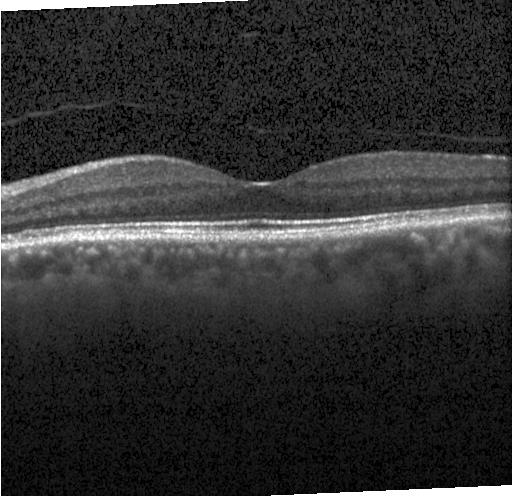

Retinal OCT cross-section
This B-scan demonstrates neither choroidal neovascularization, diabetic macular edema, nor drusen.